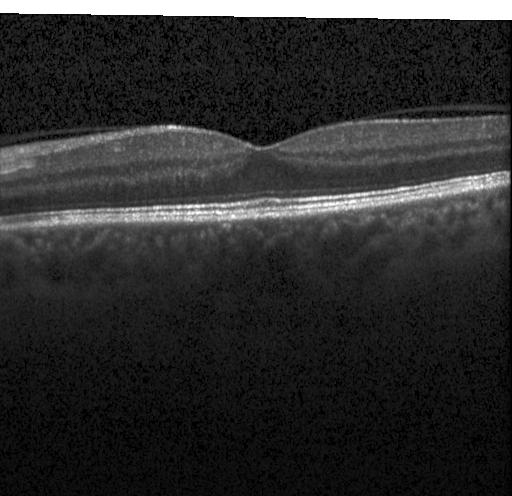

Horizontal scan through the fovea · retinal OCT B-scan · spectral-domain OCT
Assessment: no evidence of choroidal neovascularization, diabetic macular edema, or drusen.